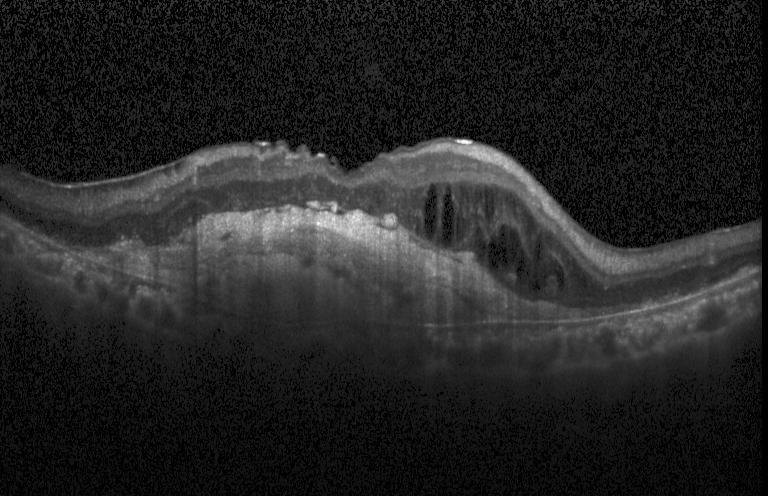 Assessment: a choroidal neovascular membrane.